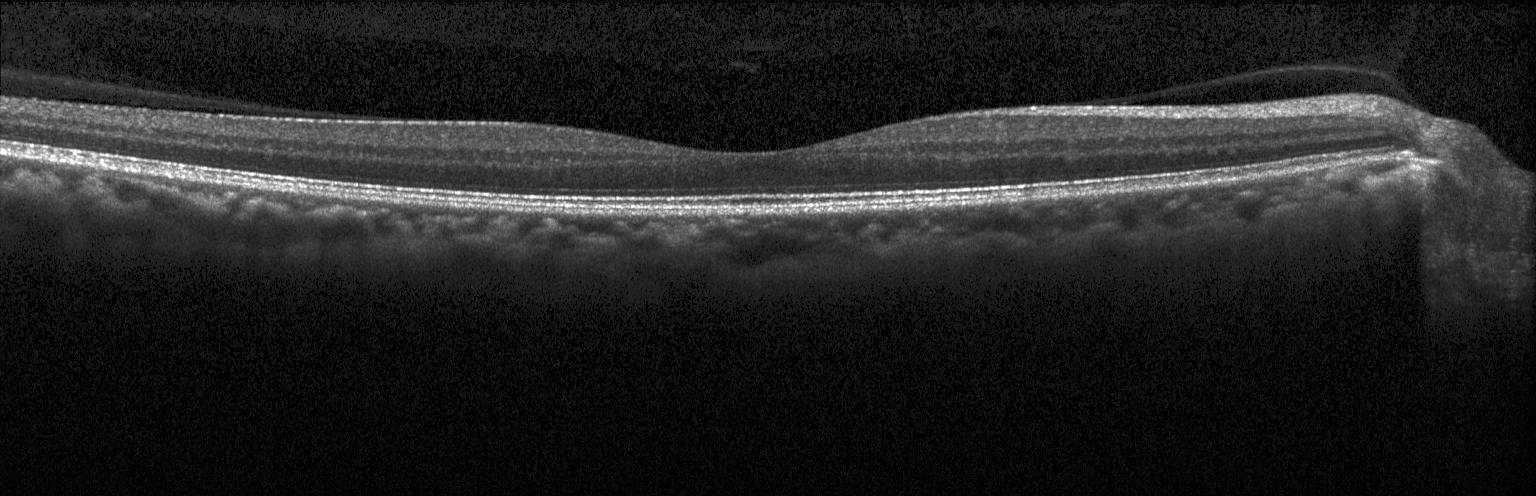
Acquired on a Heidelberg Spectralis; OCT line scan; fovea-centered.
This B-scan demonstrates no choroidal neovascularization, no diabetic macular edema, and no drusen.